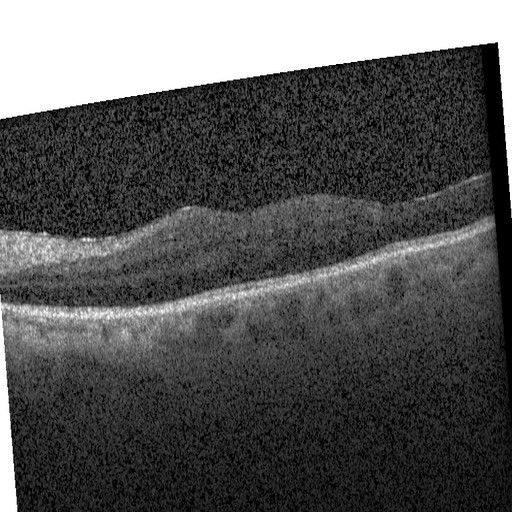
Diagnosis: diabetic macular edema.